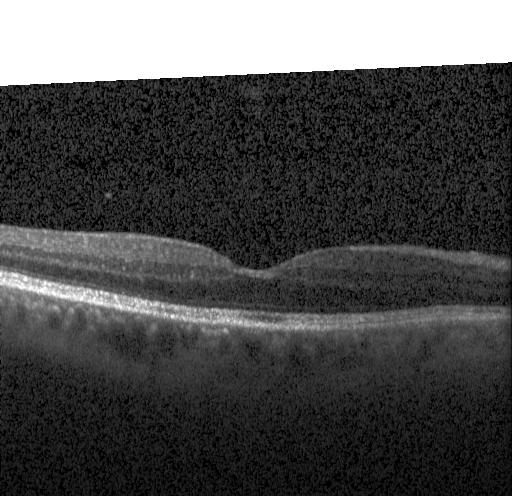
Impression: no choroidal neovascularization, no diabetic macular edema, and no drusen.